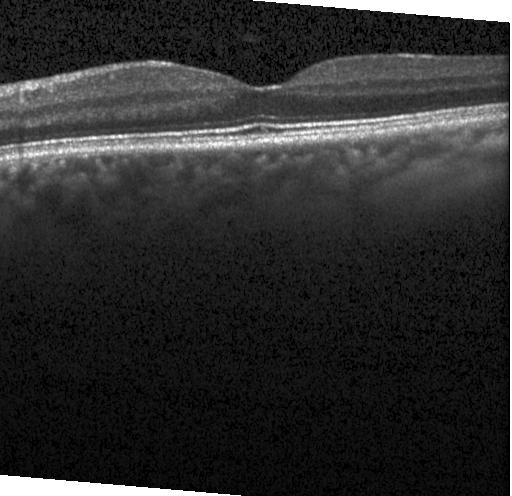

Finding: neither choroidal neovascularization, diabetic macular edema, nor drusen.